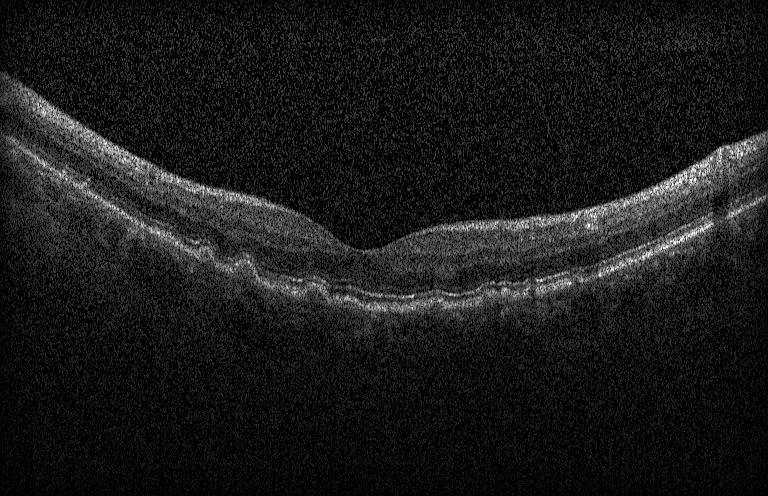

Finding: sub-RPE drusenoid deposits.